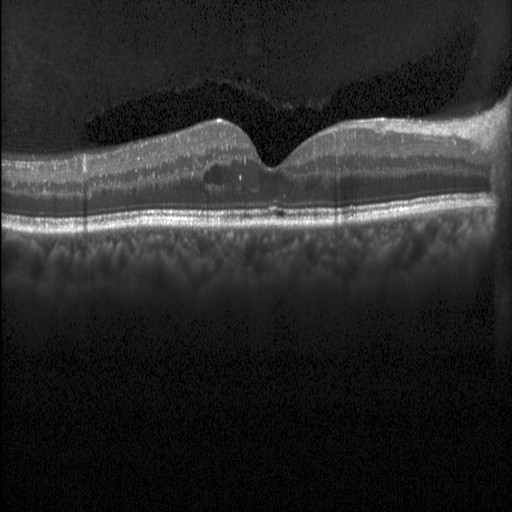
Finding: diabetic macular edema.